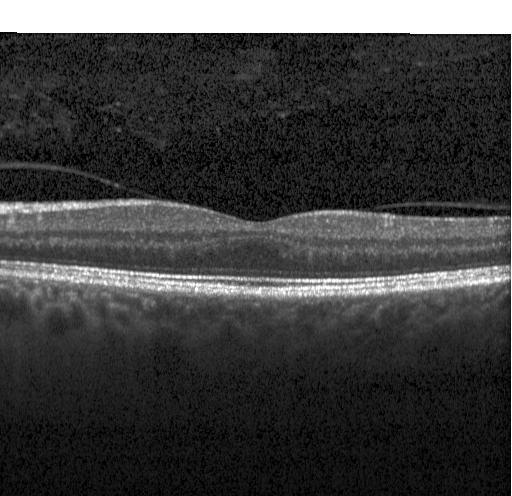
Acquired on a Heidelberg Spectralis; optical coherence tomography B-scan. Diagnosis: no evidence of choroidal neovascularization, diabetic macular edema, or drusen.